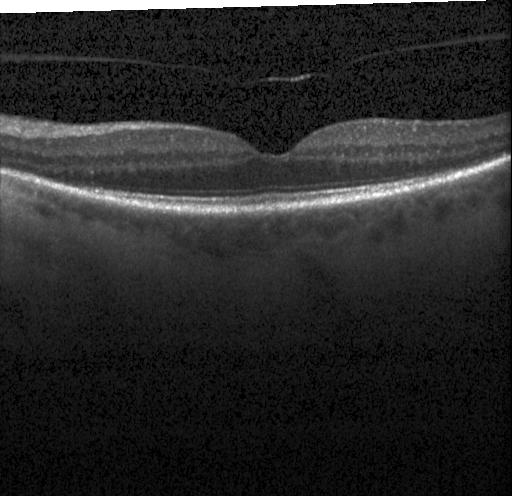 Retinal OCT cross-section showing no CNV, DME, or drusen.